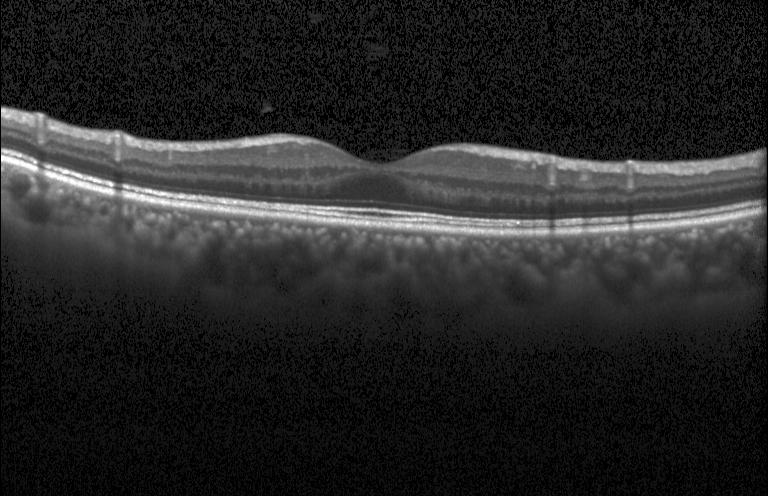 Finding: neither choroidal neovascularization, diabetic macular edema, nor drusen.